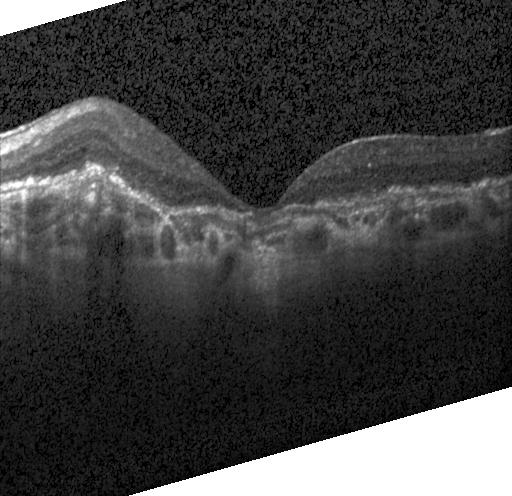

Acquired on a Heidelberg Spectralis, OCT B-scan, spectral-domain optical coherence tomography, centered on the fovea. A choroidal neovascular membrane.